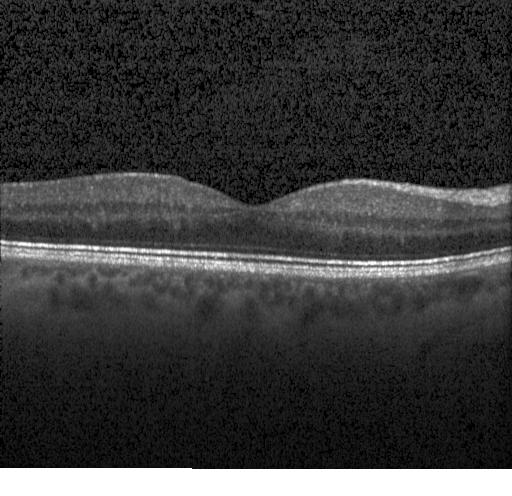

Acquired on a Heidelberg Spectralis · retinal OCT B-scan · through the macula — Finding: no evidence of choroidal neovascularization, diabetic macular edema, or drusen.